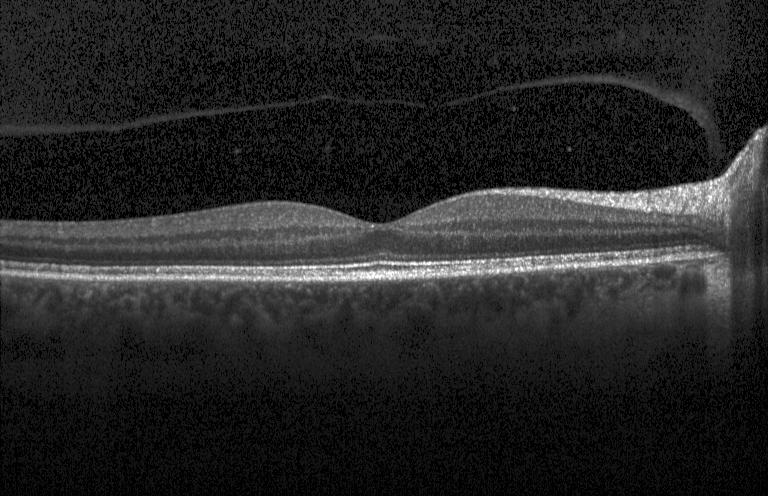
Impression: neither choroidal neovascularization, diabetic macular edema, nor drusen.